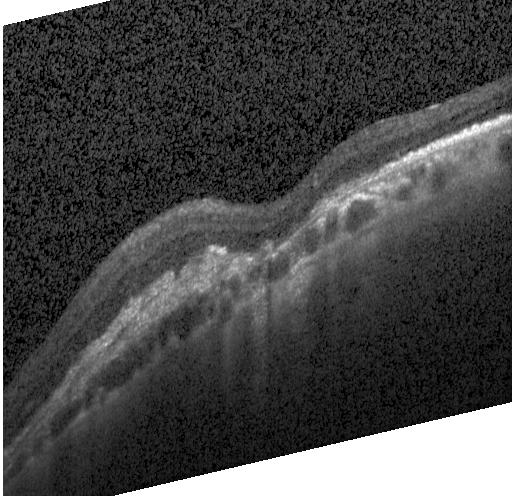 Retinal OCT cross-section.
Impression: a choroidal neovascular membrane.